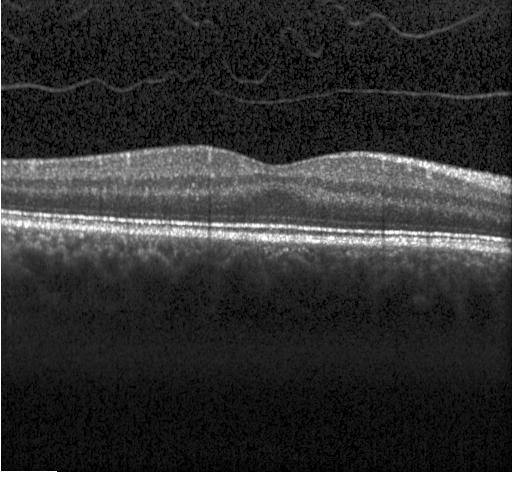
OCT line scan. Instrument: Heidelberg Spectralis.
The scan shows no evidence of CNV, DME, or drusen.